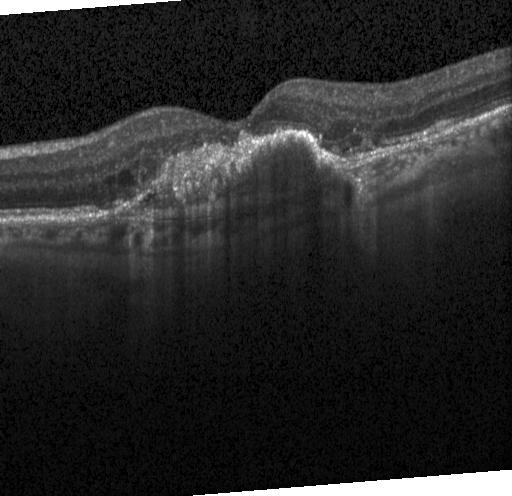
Heidelberg Spectralis. OCT B-scan. Spectral-domain optical coherence tomography.
Choroidal neovascularization.